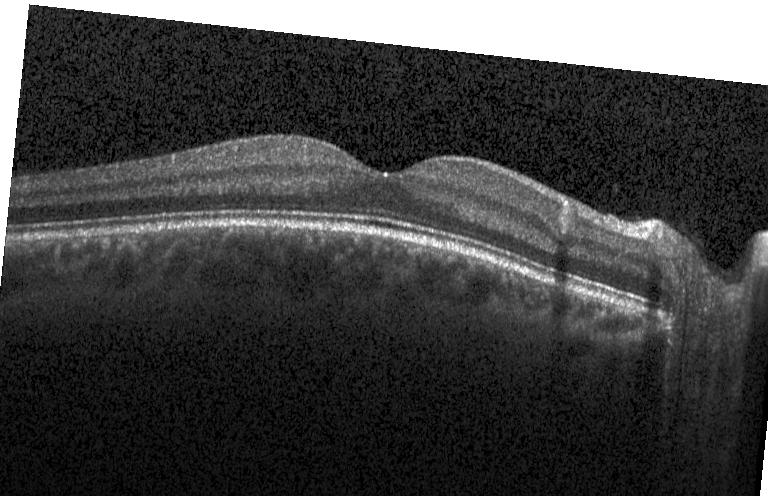 OCT B-scan showing no choroidal neovascularization, no diabetic macular edema, and no drusen.